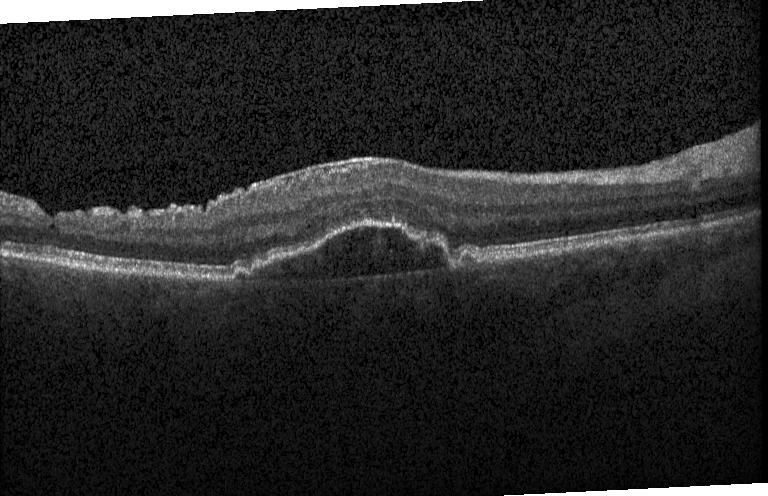

Macular OCT: a choroidal neovascular membrane.